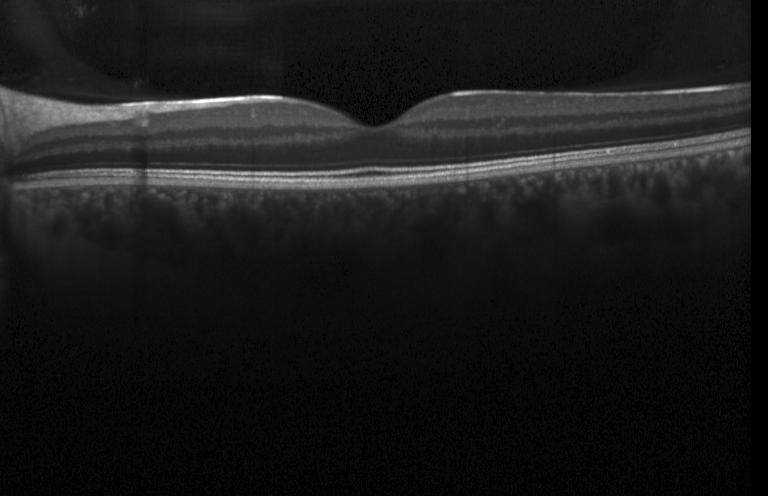
Spectral-domain OCT. Retinal OCT cross-section. Neither choroidal neovascularization, diabetic macular edema, nor drusen.